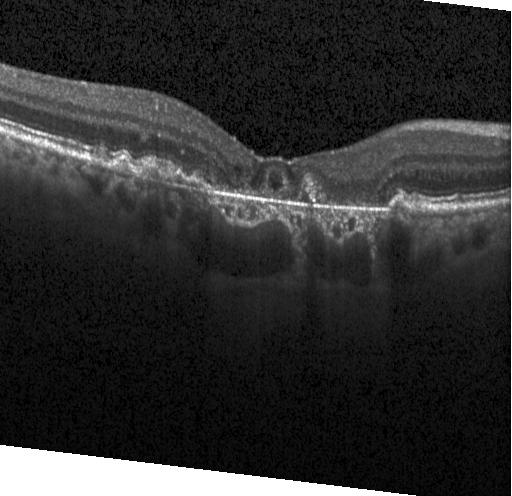 OCT scan showing a choroidal neovascular membrane.